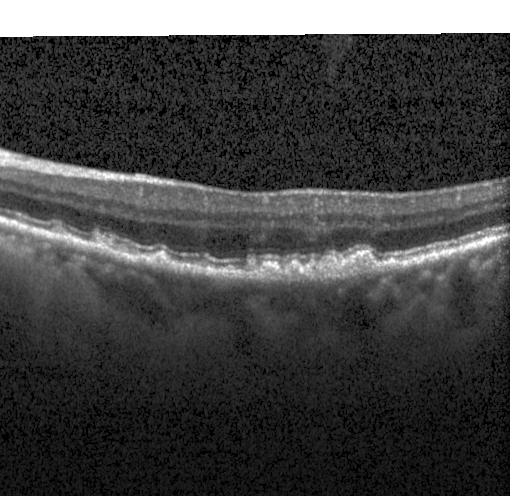
Retinal OCT B-scan — Impression: sub-RPE drusenoid deposits.